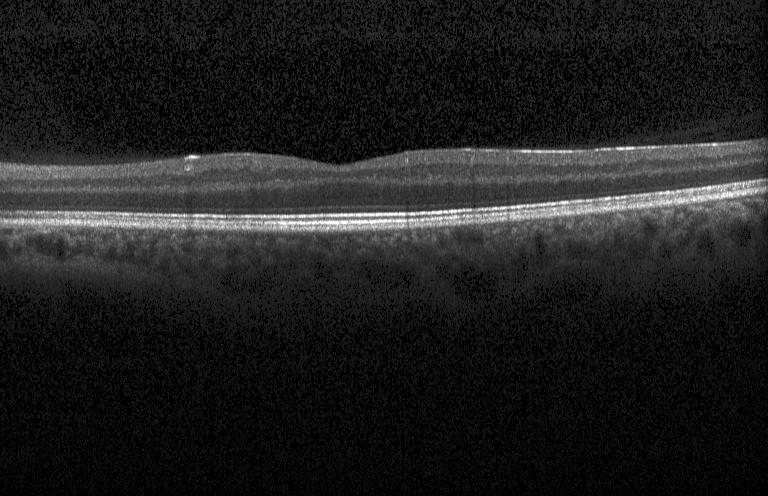

Centered on the fovea, spectral-domain OCT, retinal OCT cross-section, acquired on a Heidelberg Spectralis. The scan shows neither choroidal neovascularization, diabetic macular edema, nor drusen.